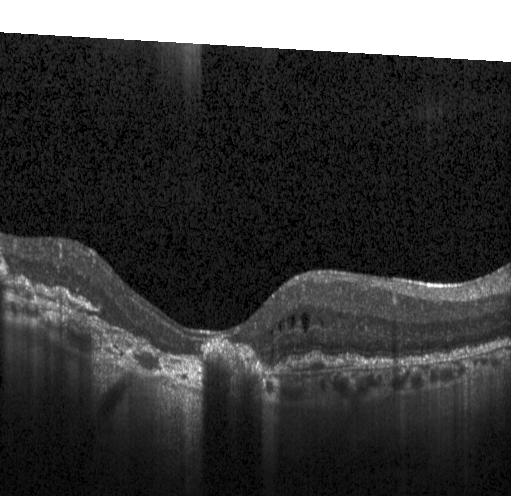 Spectral-domain optical coherence tomography · Heidelberg Spectralis · horizontal scan through the fovea · OCT B-scan
Finding: CNV.